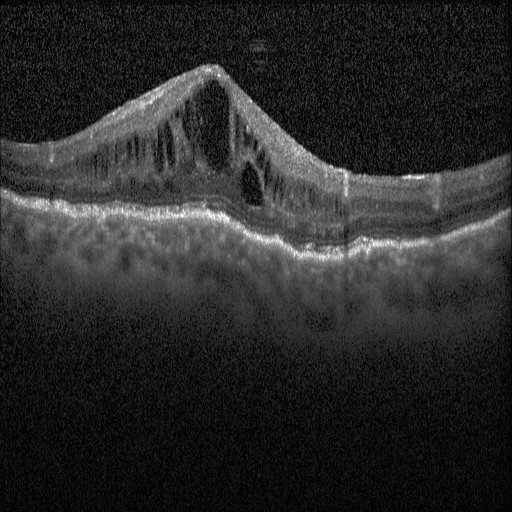 The scan shows diabetic macular edema.